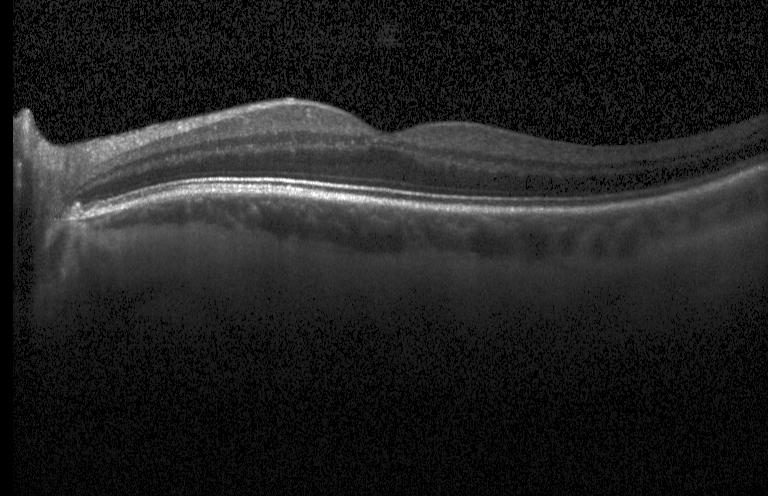

OCT B-scan. Impression: neither CNV, DME, nor drusen.